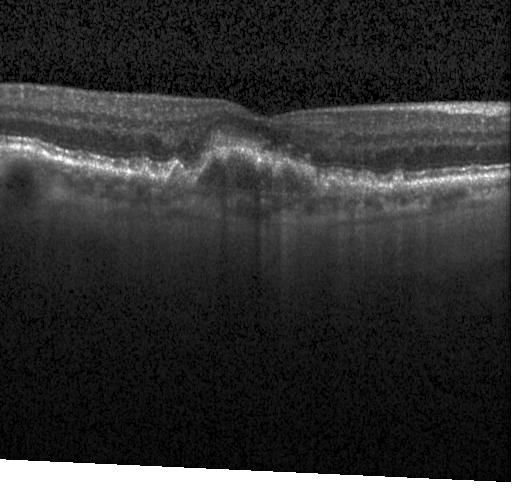
Through the macula; spectral-domain optical coherence tomography; Heidelberg Spectralis; optical coherence tomography scan.
Impression: a choroidal neovascular membrane.